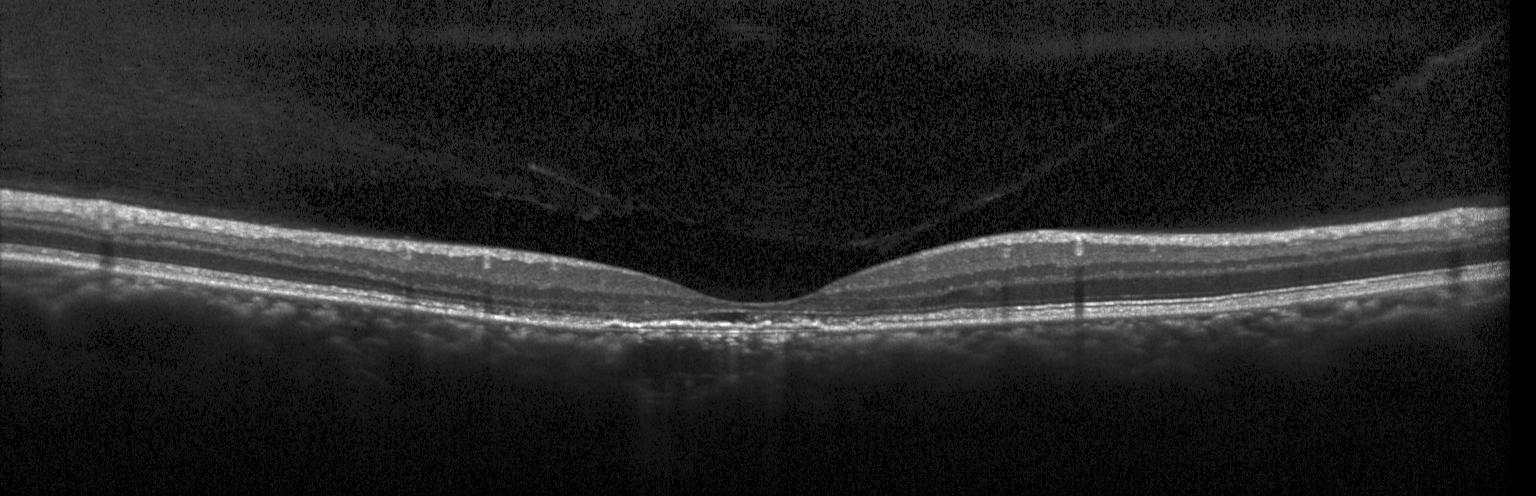 Finding: a choroidal neovascular membrane.